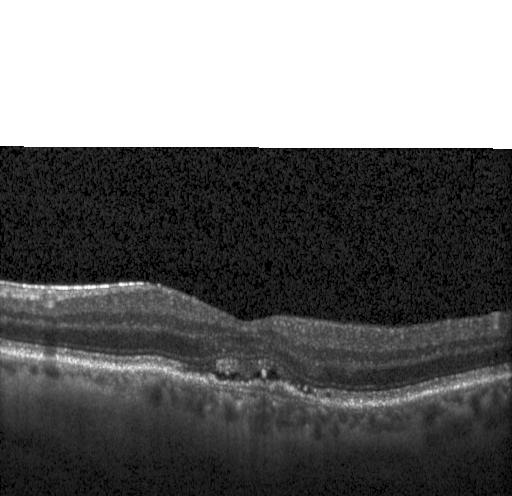

Finding: choroidal neovascularization.